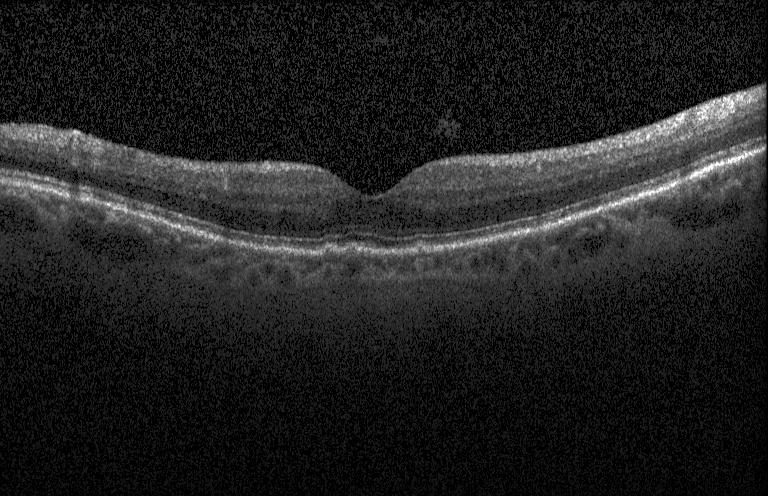

Retinal OCT cross-section.
Diagnosis: multiple drusen.